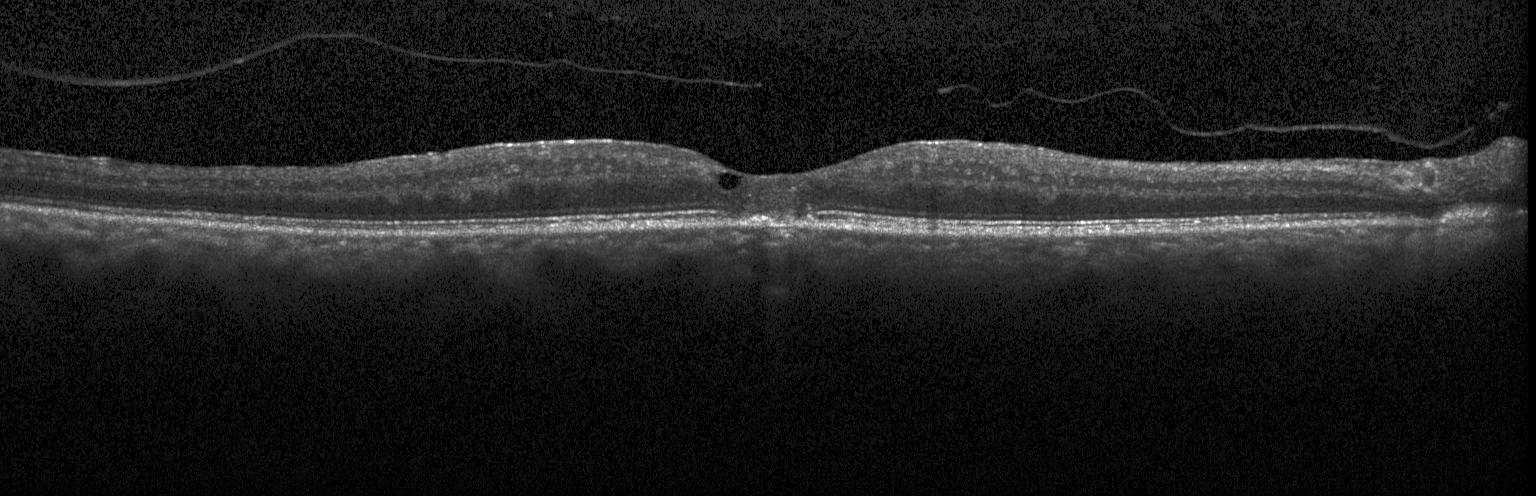
Diagnosis: DME.